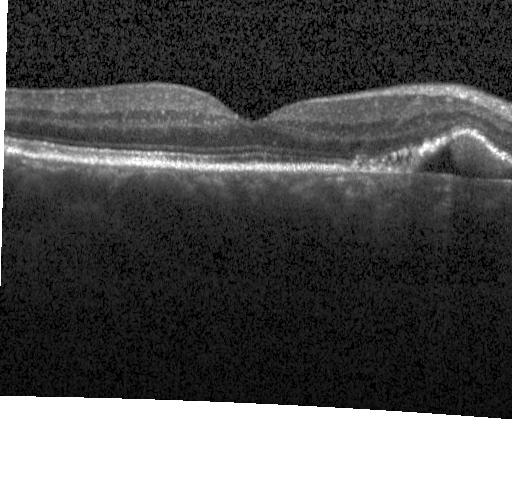 SD-OCT. Instrument: Heidelberg Spectralis. Horizontal scan through the fovea. Optical coherence tomography B-scan — The scan shows choroidal neovascularization (CNV).